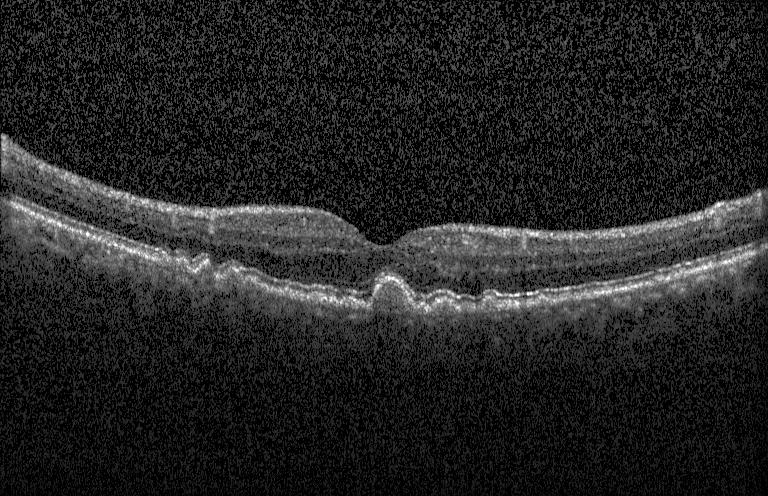 Impression: sub-RPE drusenoid deposits.